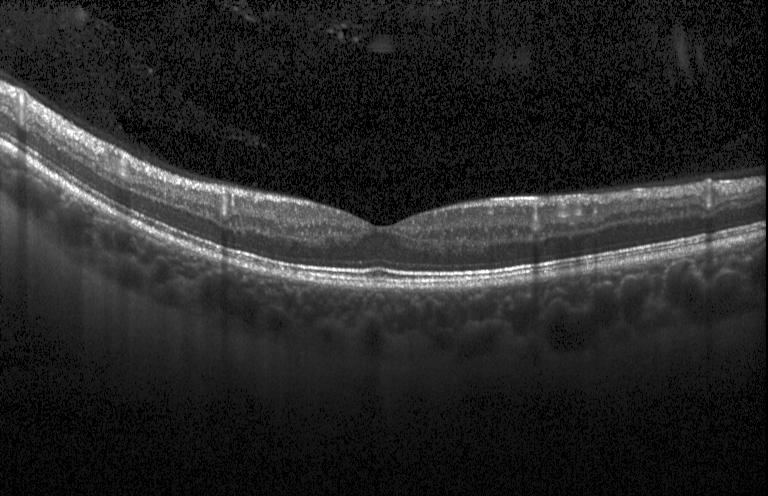 Spectral-domain OCT B-scan: no evidence of CNV, DME, or drusen.